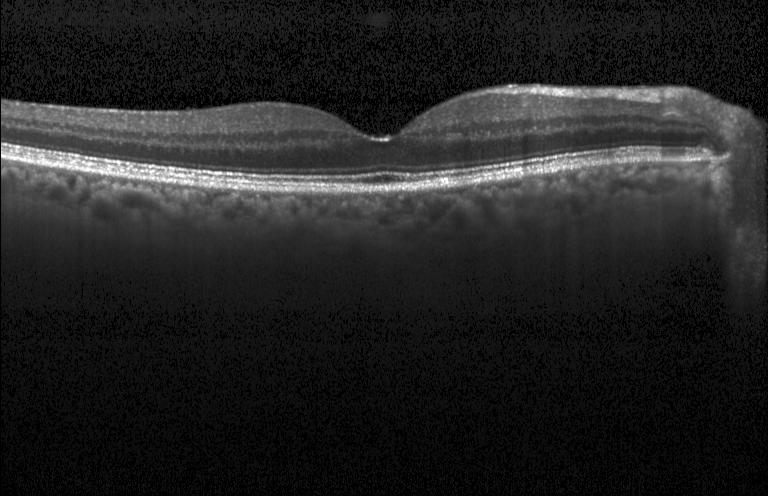 Macular OCT: neither choroidal neovascularization, diabetic macular edema, nor drusen.